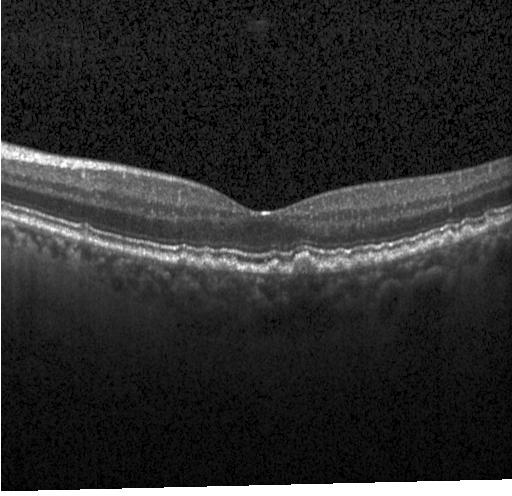 Fovea-centered, Heidelberg Spectralis, retinal OCT cross-section.
Diagnosis: multiple drusen.